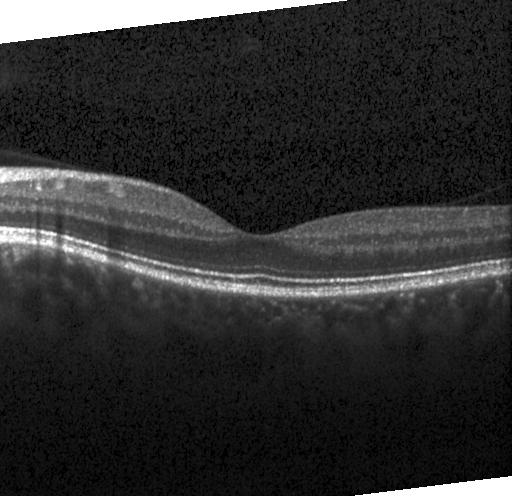
Finding: neither choroidal neovascularization, diabetic macular edema, nor drusen.